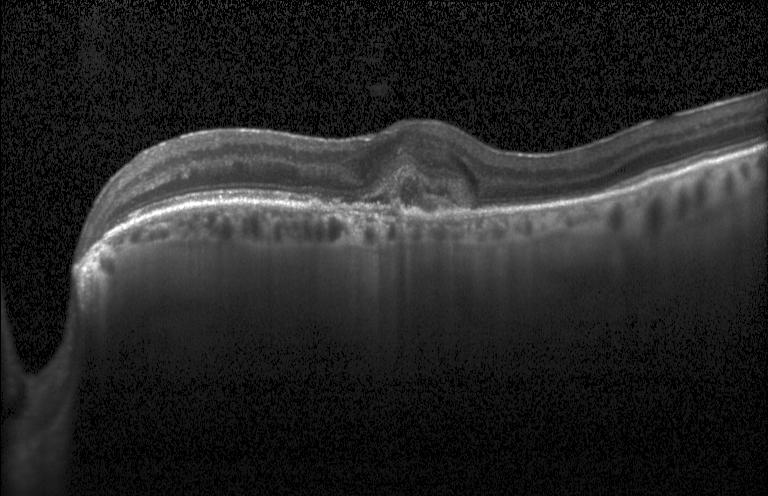 Horizontal scan through the fovea. OCT B-scan. Spectral-domain OCT
Finding: a choroidal neovascular membrane.